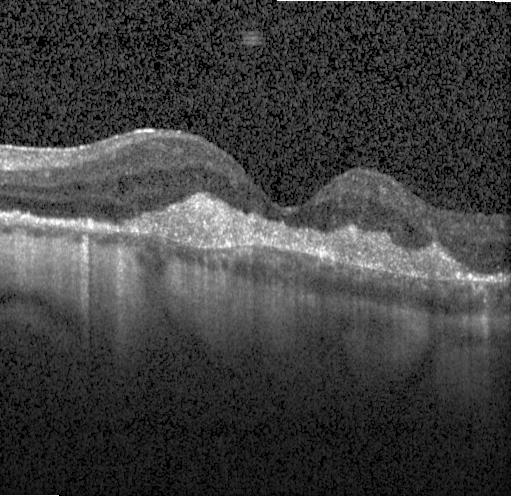 Finding: a choroidal neovascular membrane.